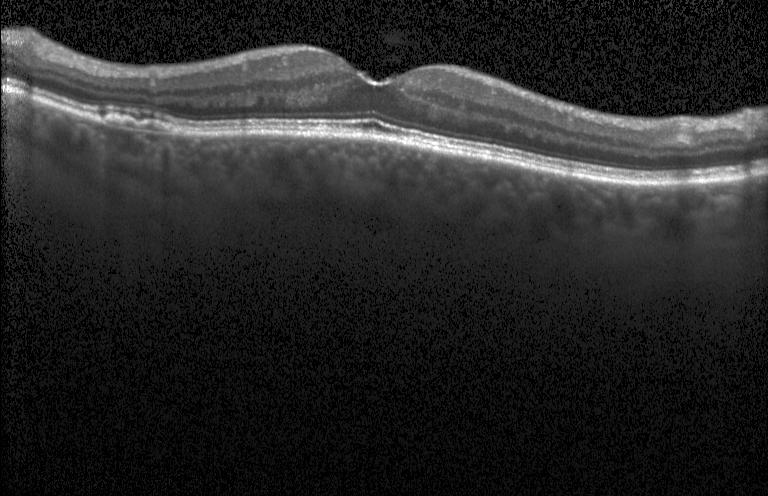

Macular OCT: CNV.